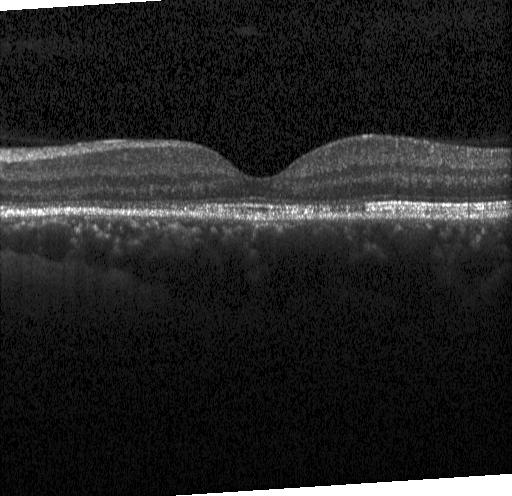
Macular OCT demonstrating no choroidal neovascularization, diabetic macular edema, or drusen.